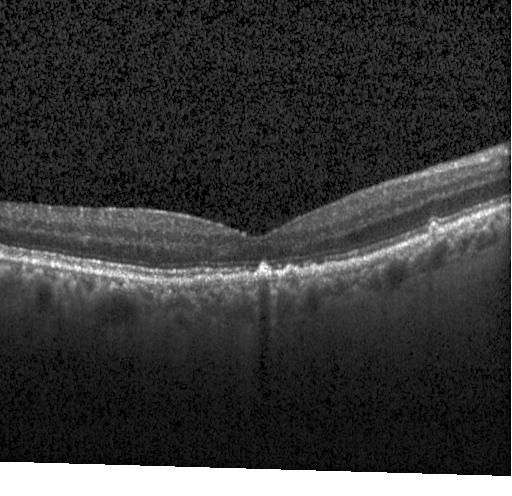

Finding: multiple drusen.